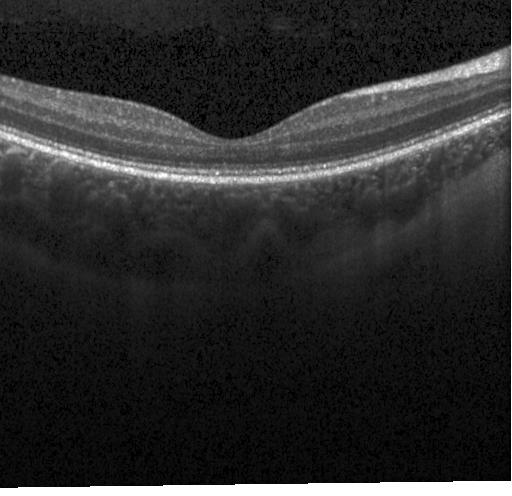 Through the macula, optical coherence tomography B-scan, Heidelberg Spectralis OCT system
Impression: no choroidal neovascularization, diabetic macular edema, or drusen.